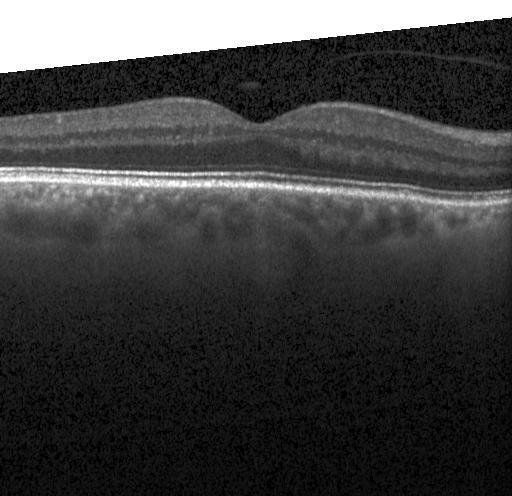 OCT B-scan showing no evidence of CNV, DME, or drusen.